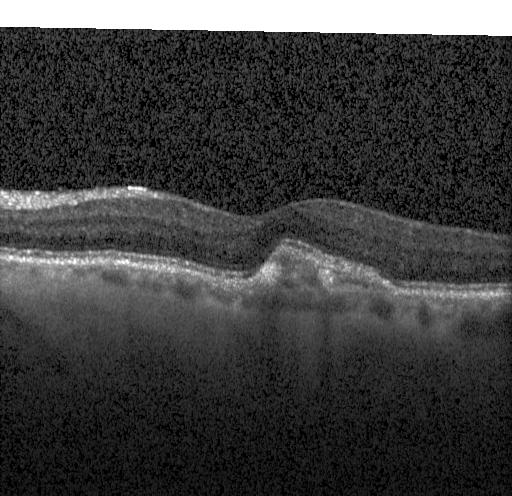

OCT B-scan showing a choroidal neovascular membrane.